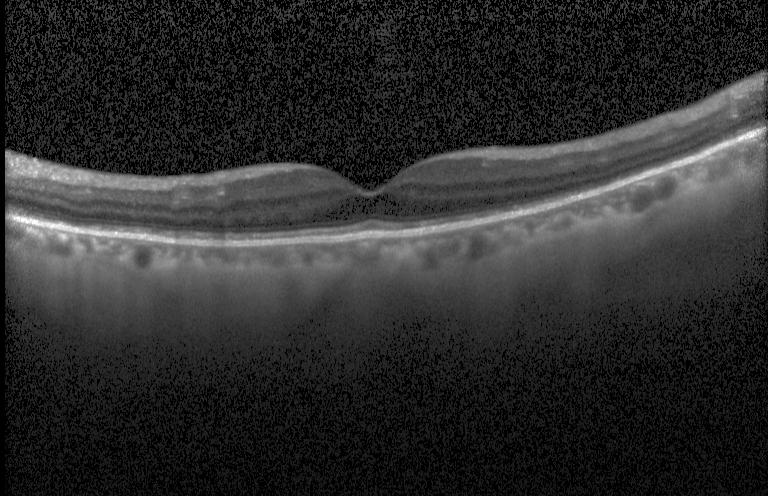
SD-OCT · Heidelberg Spectralis · OCT line scan · centered on the fovea. Dx: no evidence of choroidal neovascularization, diabetic macular edema, or drusen.